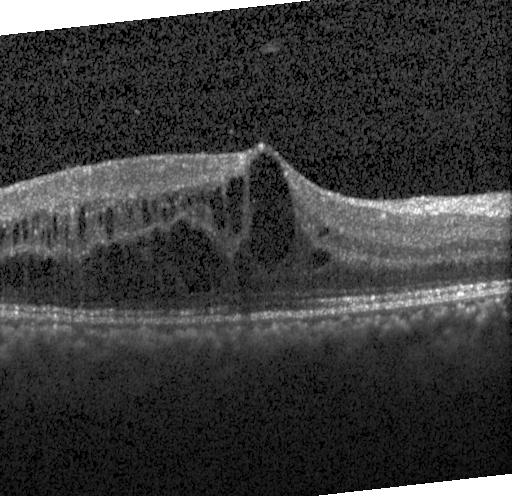 Diagnosis: DME.